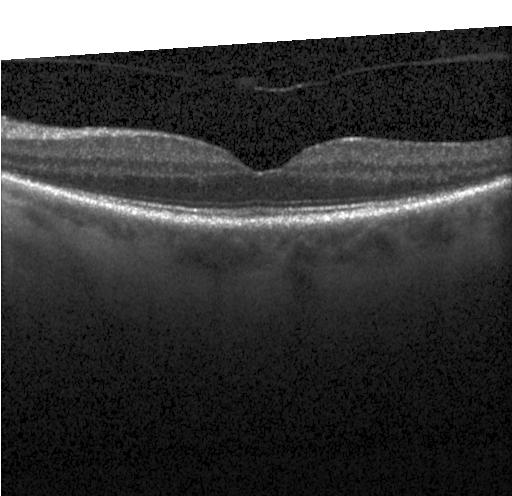 Fovea-centered. OCT B-scan. Heidelberg Spectralis OCT system
Finding: neither choroidal neovascularization, diabetic macular edema, nor drusen.